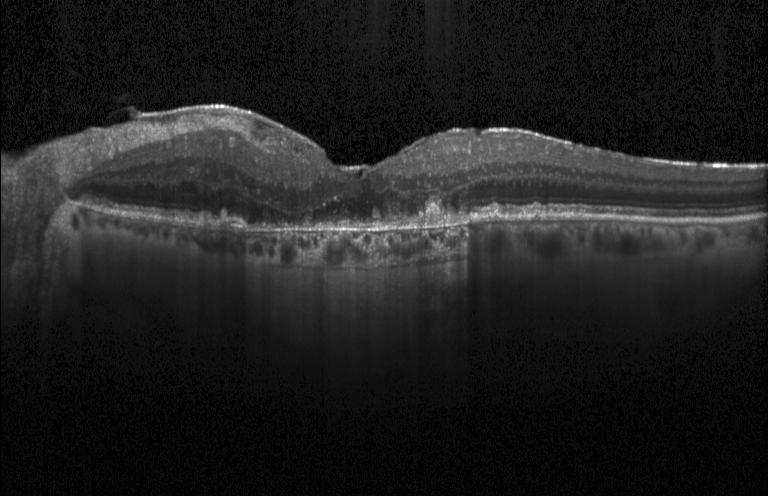

Optical coherence tomography B-scan.
Impression: a choroidal neovascular membrane.